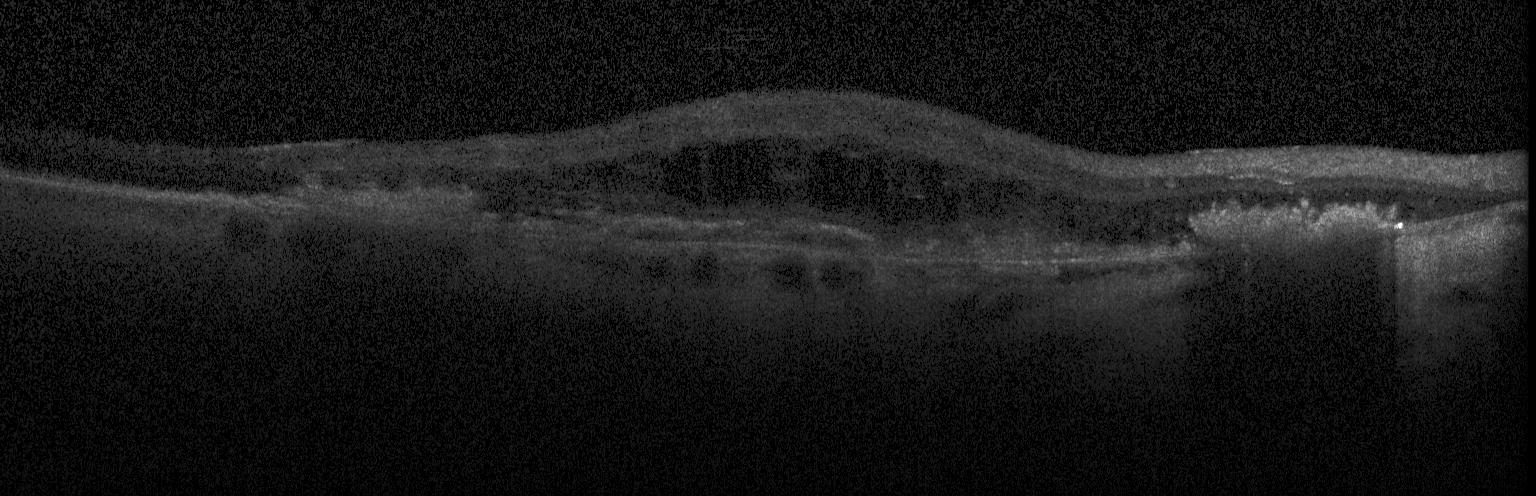

Acquired on a Heidelberg Spectralis, OCT B-scan
The scan shows a choroidal neovascular membrane.